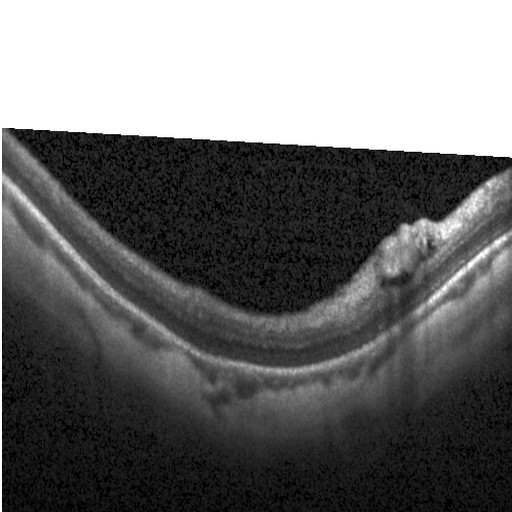 Fovea-centered. Spectral-domain OCT. Retinal OCT cross-section. Heidelberg Spectralis OCT system
OCT finding: diabetic macular edema (DME).